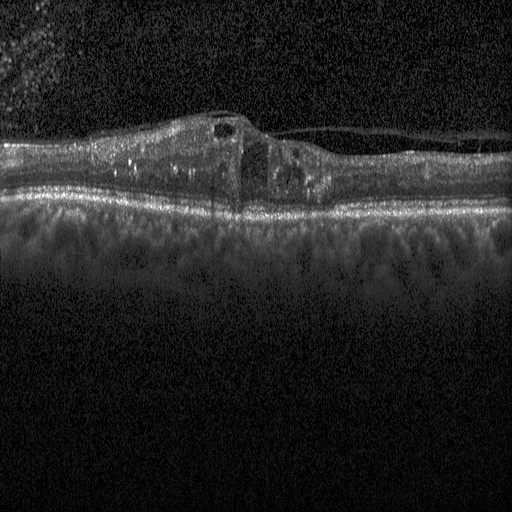 OCT line scan · Heidelberg Spectralis OCT system
This B-scan demonstrates diabetic macular edema.